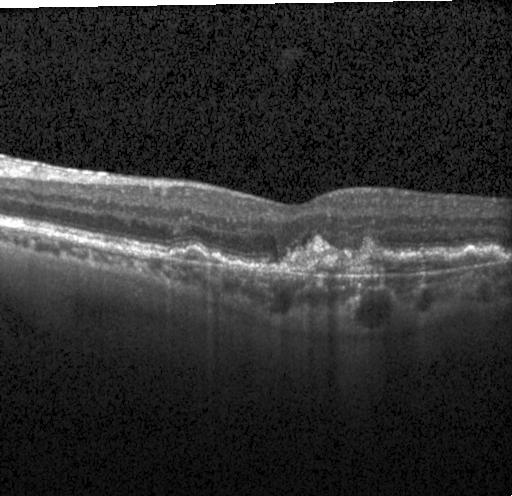

Optical coherence tomography B-scan
Finding: choroidal neovascularization.